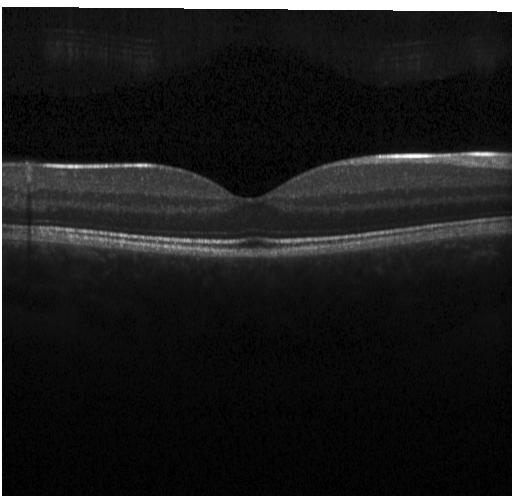
OCT B-scan showing no choroidal neovascularization, diabetic macular edema, or drusen.